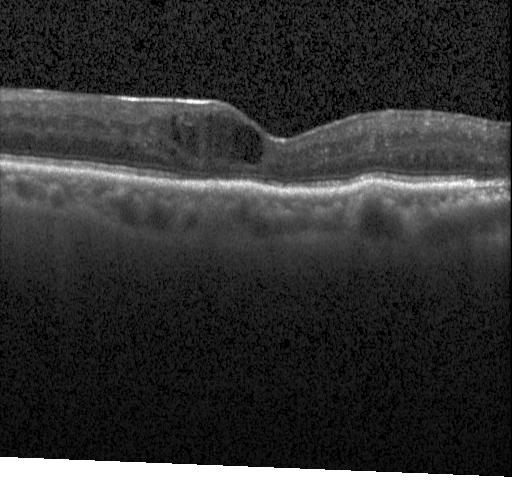
Dx: diabetic macular edema (DME).